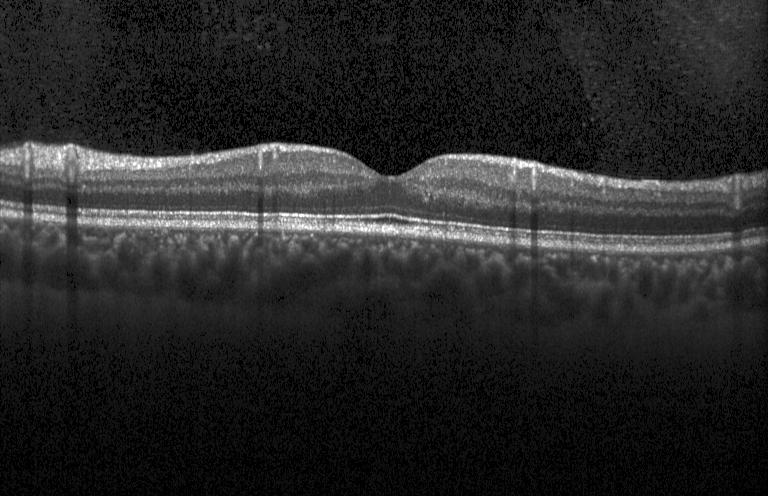 Horizontal scan through the fovea · OCT line scan.
Assessment: no choroidal neovascularization, no diabetic macular edema, and no drusen.